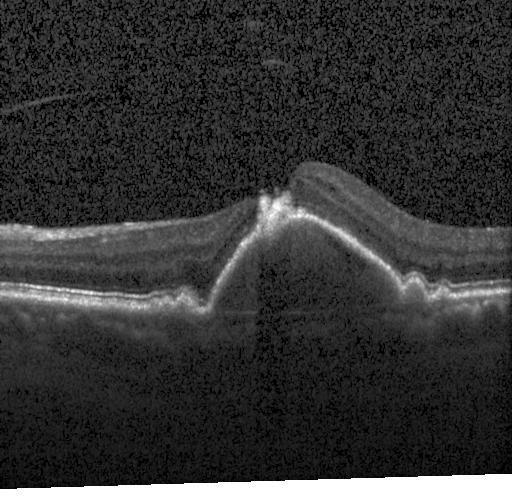
Impression: choroidal neovascularization.